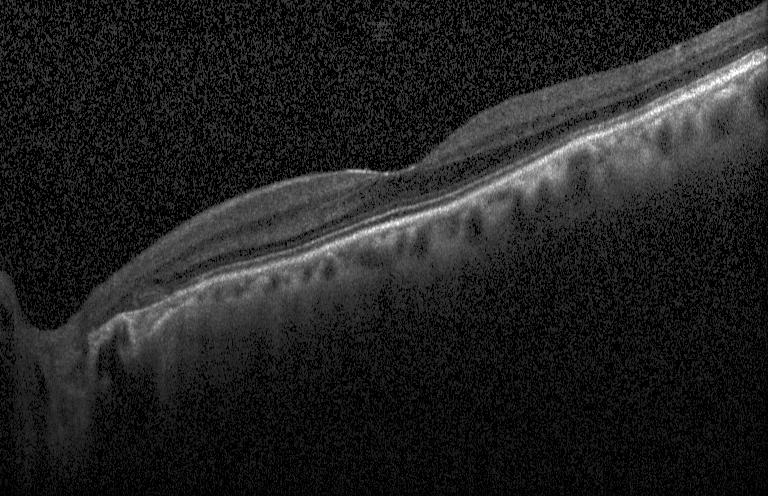 Macular OCT: no choroidal neovascularization, no diabetic macular edema, and no drusen.